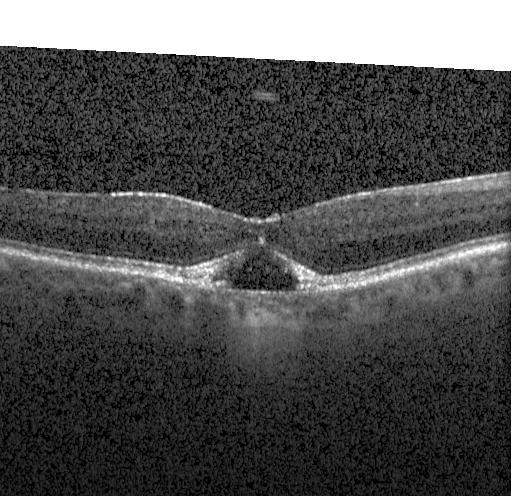
Spectral-domain OCT, optical coherence tomography B-scan, Heidelberg Spectralis, horizontal scan through the fovea. The scan shows a choroidal neovascular membrane.